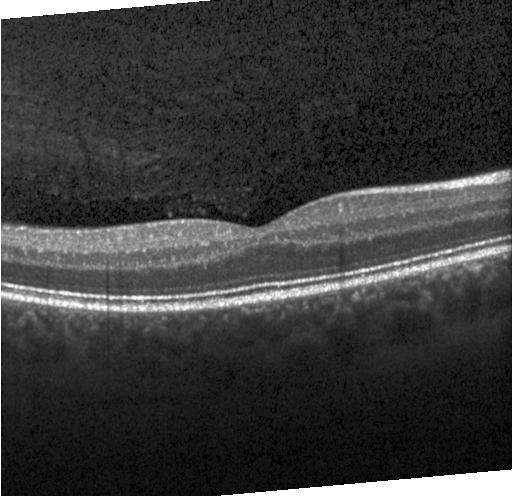 Spectral-domain OCT, acquired on a Heidelberg Spectralis, OCT B-scan. Macular OCT: neither CNV, DME, nor drusen.